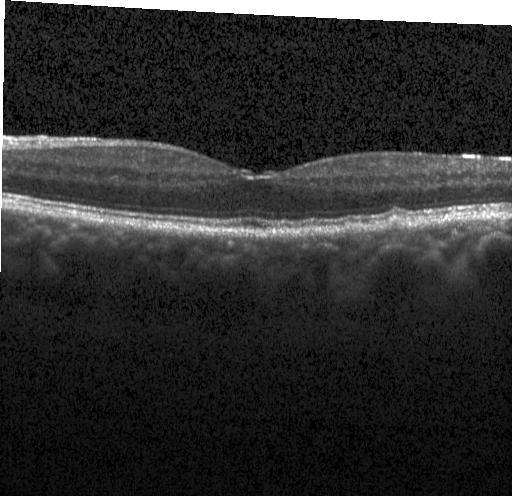

The scan shows multiple drusen.